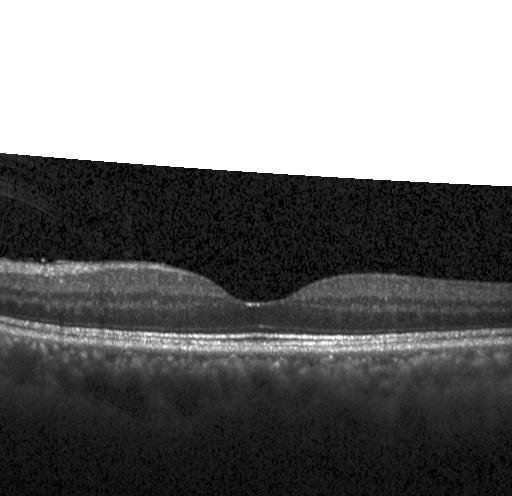 Optical coherence tomography B-scan; SD-OCT; through the macula; acquired on a Heidelberg Spectralis. This B-scan demonstrates no choroidal neovascularization, diabetic macular edema, or drusen.